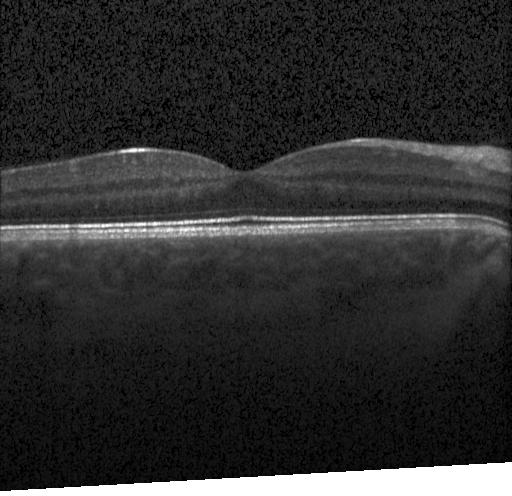

Retinal OCT cross-section. Heidelberg Spectralis.
The scan shows no CNV, DME, or drusen.